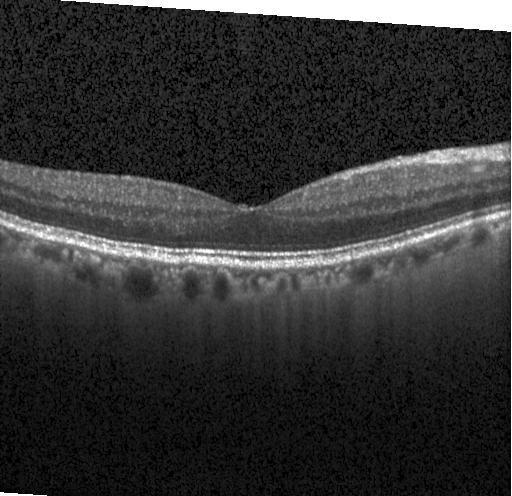 Instrument: Heidelberg Spectralis, retinal OCT B-scan.
Impression: neither choroidal neovascularization, diabetic macular edema, nor drusen.